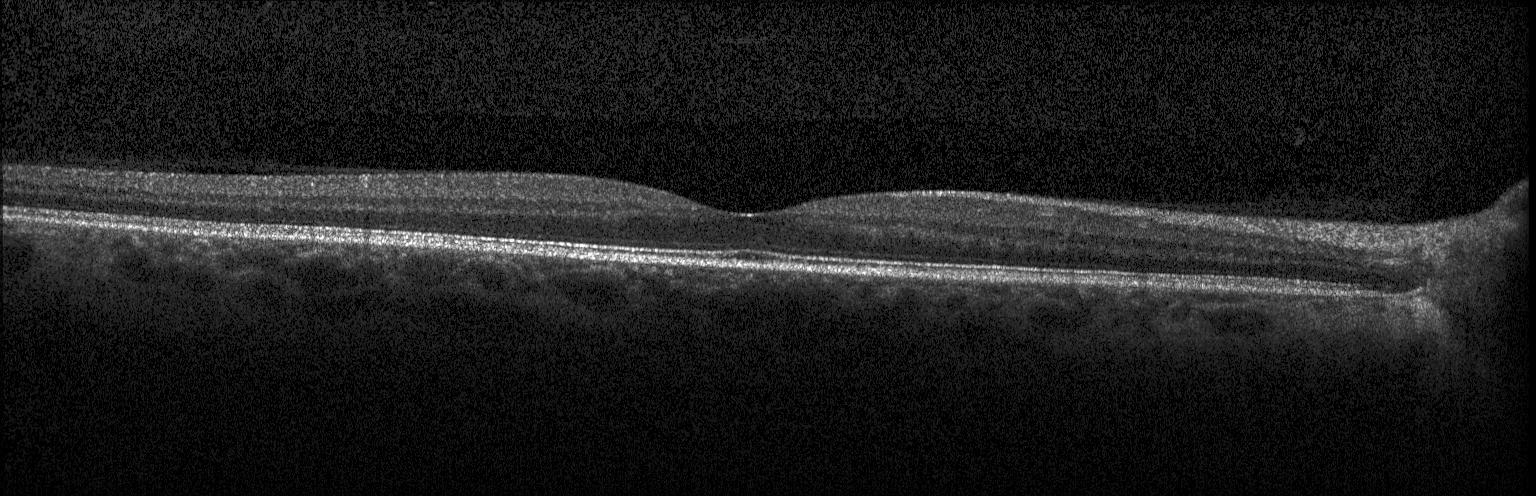 Finding: no CNV, DME, or drusen.